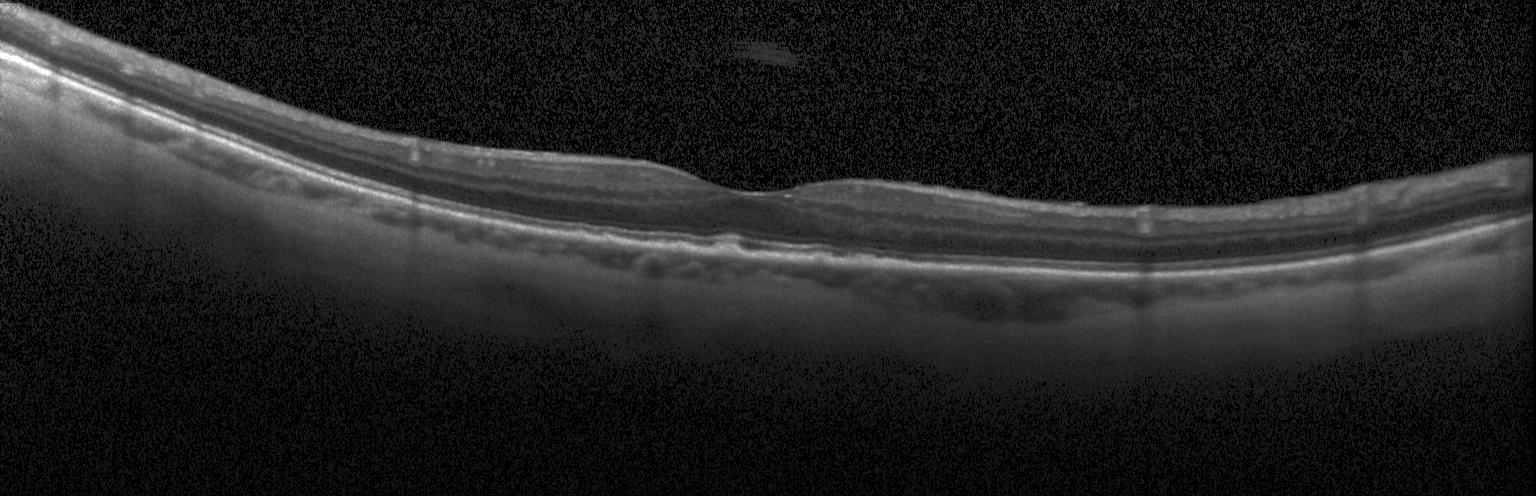 Impression: sub-RPE drusenoid deposits.